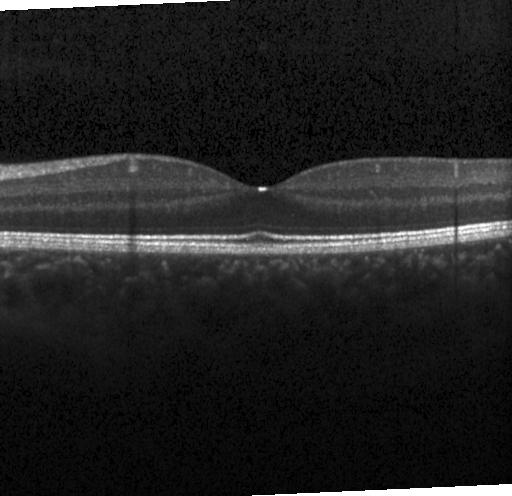

Fovea-centered, optical coherence tomography scan, instrument: Heidelberg Spectralis
Impression: no evidence of CNV, DME, or drusen.